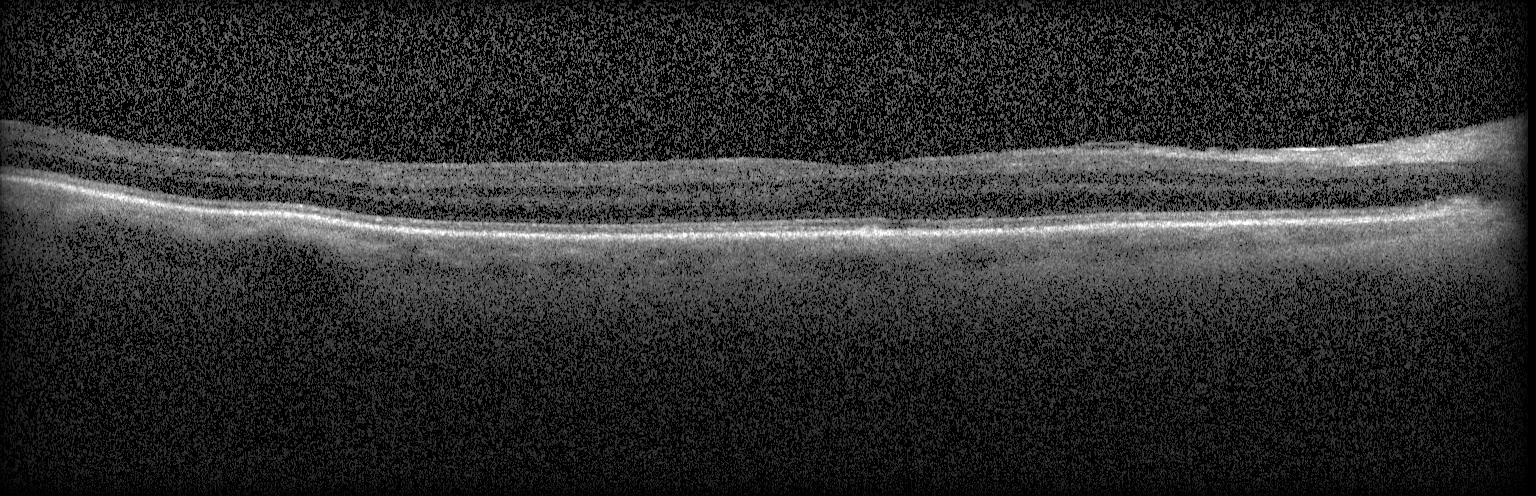 Finding: no CNV, no DME, and no drusen.